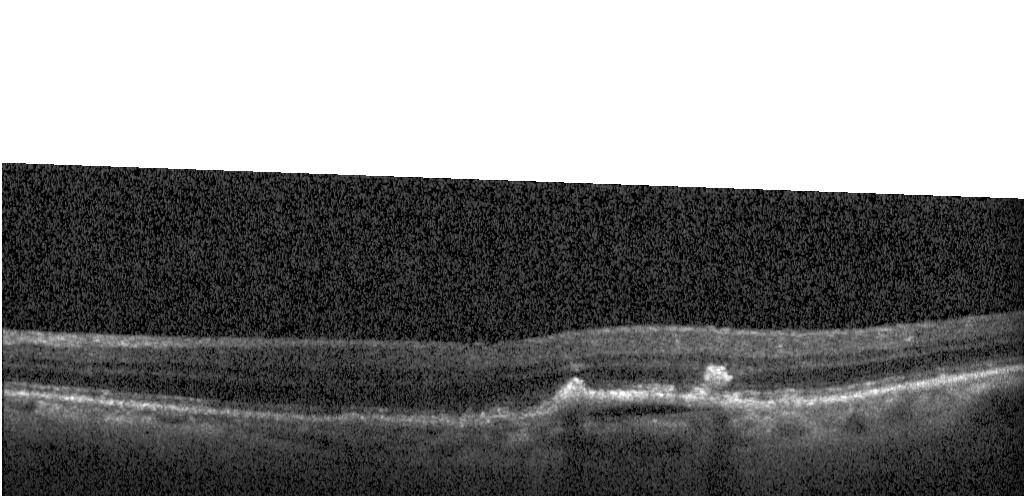 Optical coherence tomography B-scan.
Finding: a choroidal neovascular membrane.